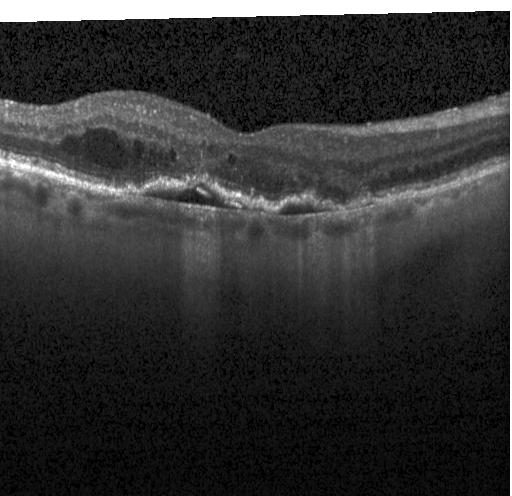 Retinal OCT cross-section; spectral-domain optical coherence tomography; through the macula; Heidelberg Spectralis
This B-scan demonstrates choroidal neovascularization.